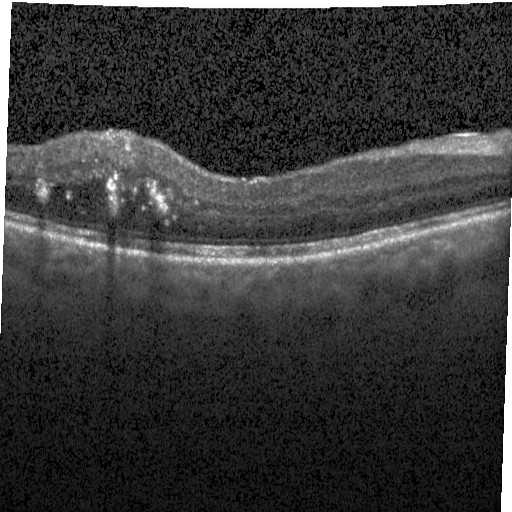

Finding: diabetic macular edema.